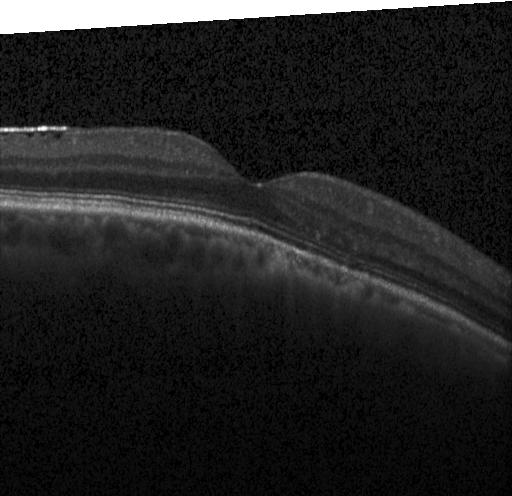

Diagnosis: no CNV, no DME, and no drusen.